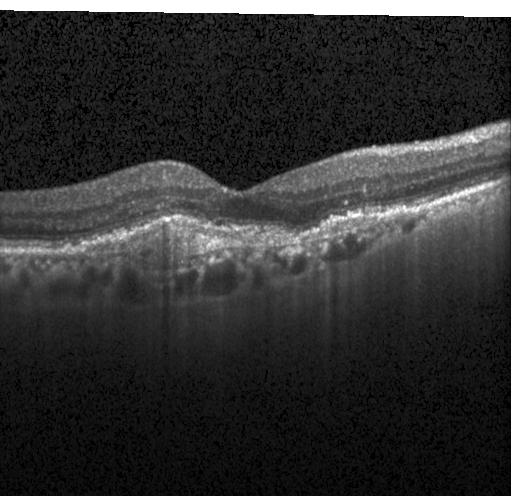

The scan shows a choroidal neovascular membrane.